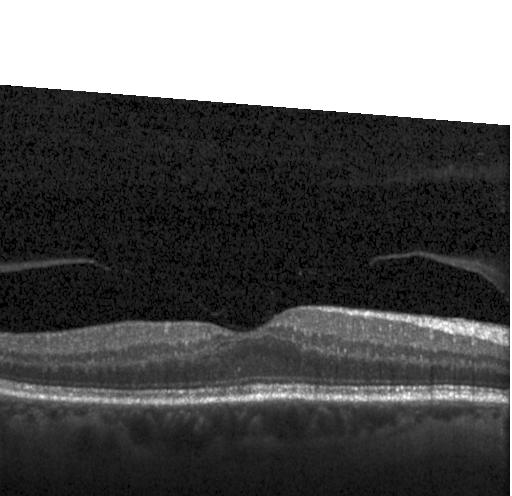 Optical coherence tomography B-scan
Impression: no evidence of choroidal neovascularization, diabetic macular edema, or drusen.